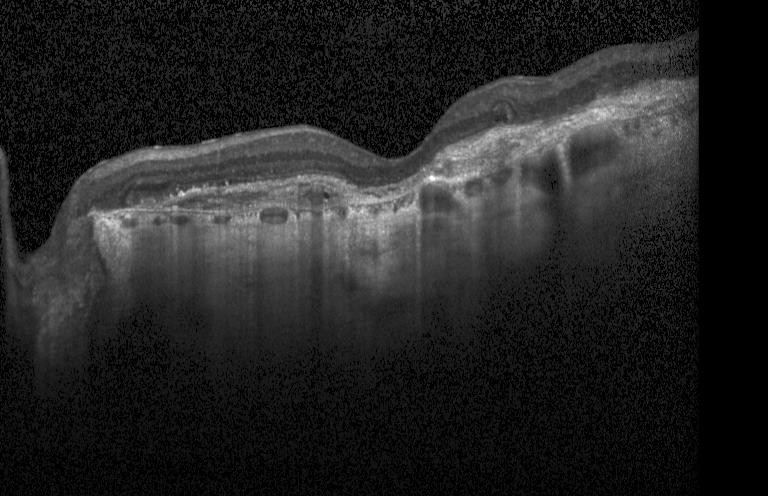

OCT B-scan.
Dx: choroidal neovascularization (CNV).